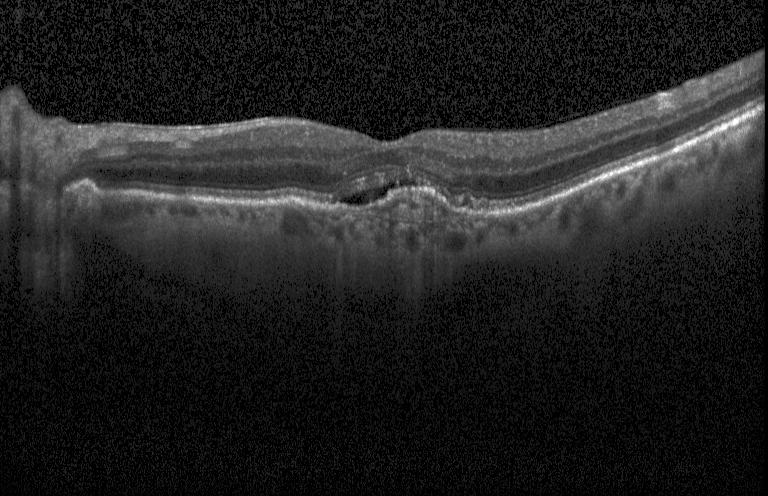
SD-OCT, macular scan, retinal OCT B-scan, instrument: Heidelberg Spectralis — Impression: a choroidal neovascular membrane.